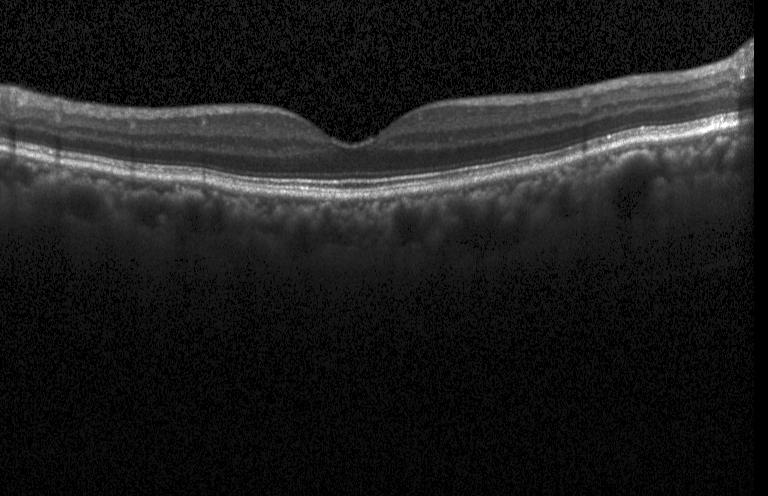
No choroidal neovascularization, no diabetic macular edema, and no drusen.